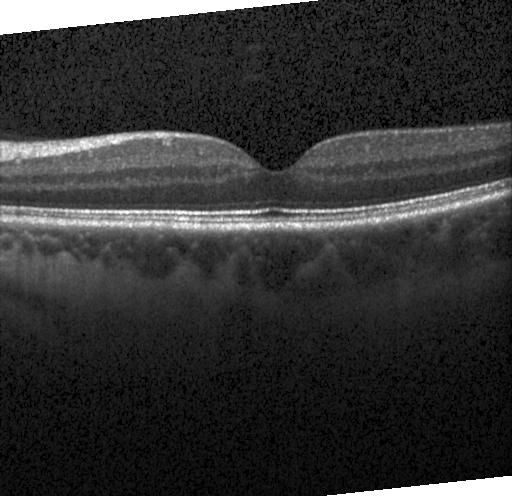 Macular OCT demonstrating neither choroidal neovascularization, diabetic macular edema, nor drusen.